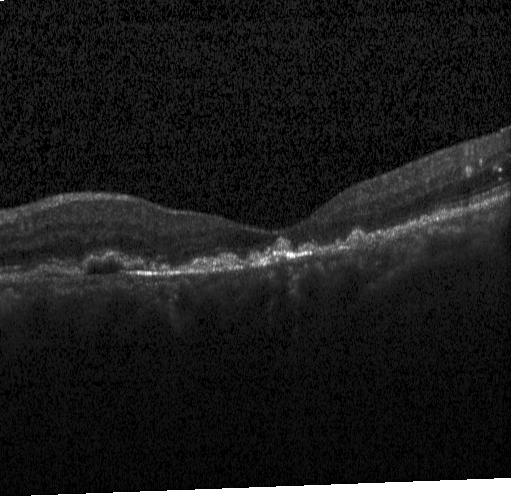
OCT B-scan. Impression: choroidal neovascularization (CNV).